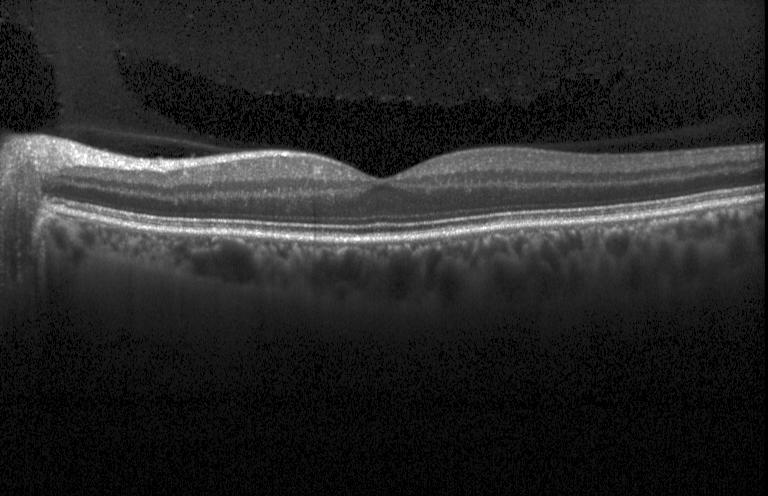 Spectral-domain OCT. OCT B-scan. Centered on the fovea
Assessment: no evidence of CNV, DME, or drusen.